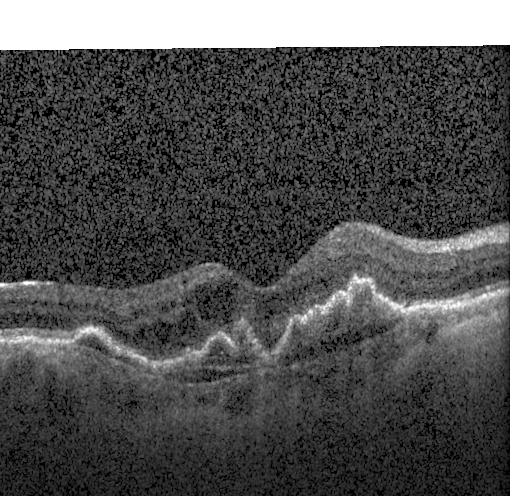
OCT B-scan showing a choroidal neovascular membrane.